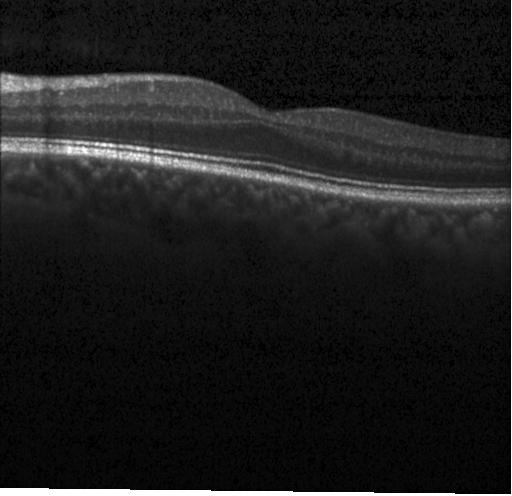

OCT B-scan showing no choroidal neovascularization, no diabetic macular edema, and no drusen.